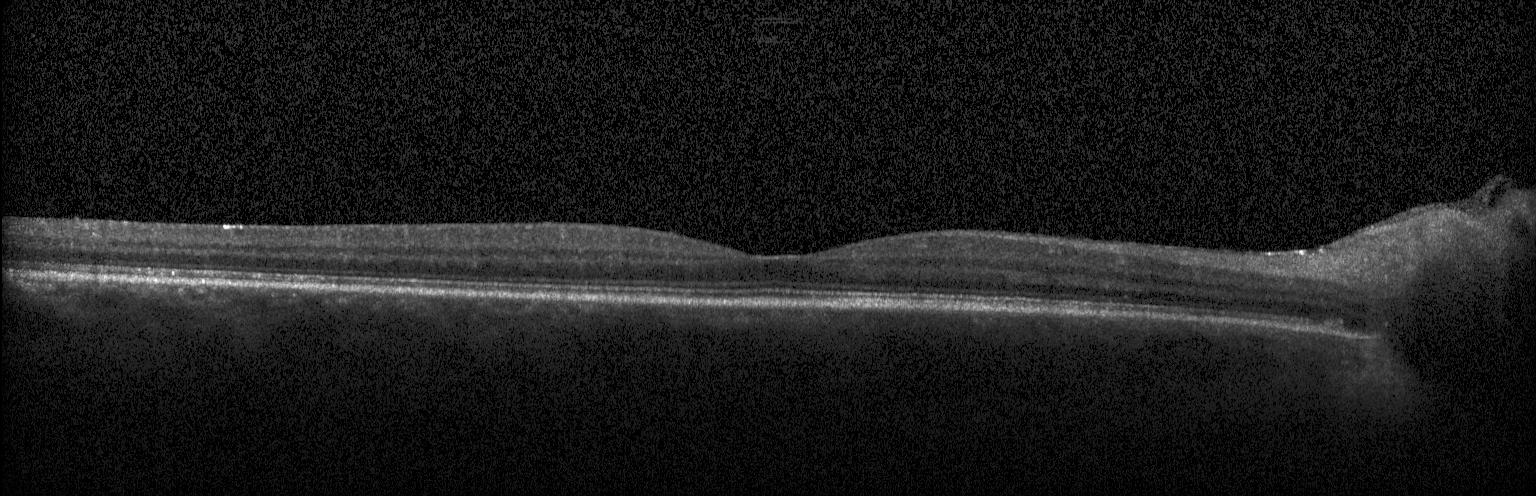
OCT scan showing no choroidal neovascularization, no diabetic macular edema, and no drusen.